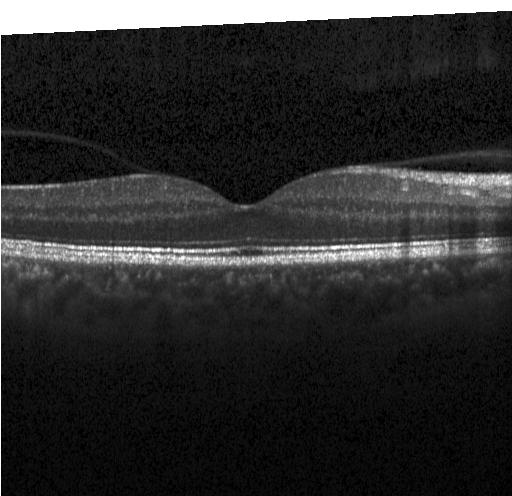 Neither CNV, DME, nor drusen.